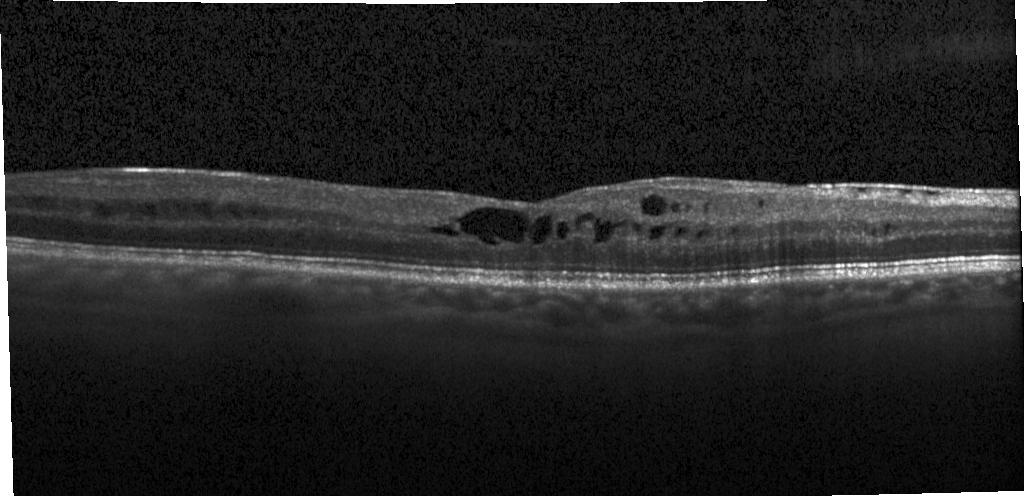
Acquired on a Heidelberg Spectralis; optical coherence tomography B-scan; through the macula; spectral-domain optical coherence tomography. Finding: DME.